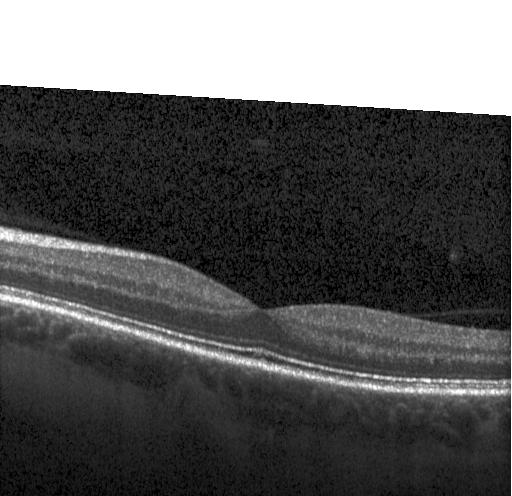

OCT scan showing no evidence of choroidal neovascularization, diabetic macular edema, or drusen.